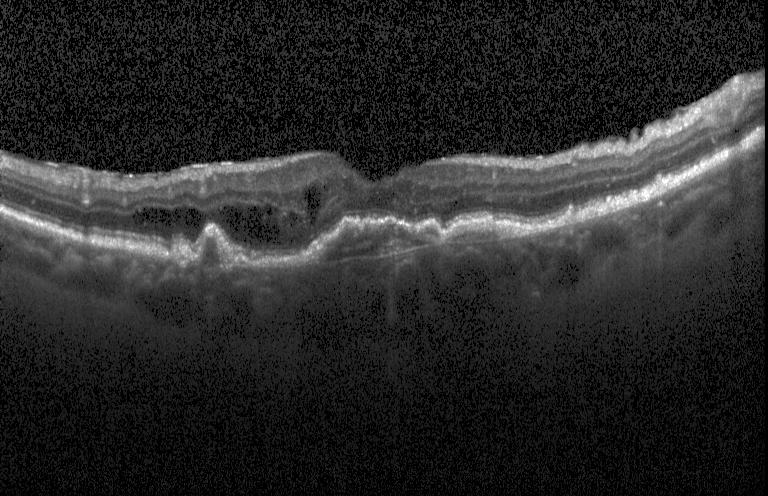

Fovea-centered. OCT B-scan. Spectral-domain OCT. Heidelberg Spectralis OCT system.
Diagnosis: a choroidal neovascular membrane.